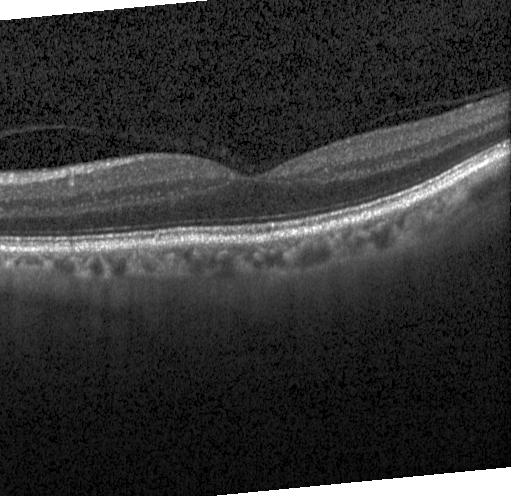
Optical coherence tomography B-scan. Impression: neither CNV, DME, nor drusen.